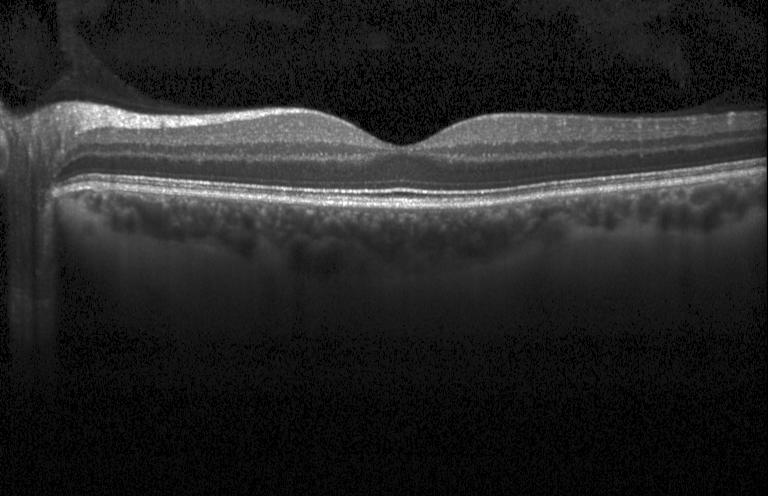
OCT line scan. Finding: no choroidal neovascularization, diabetic macular edema, or drusen.